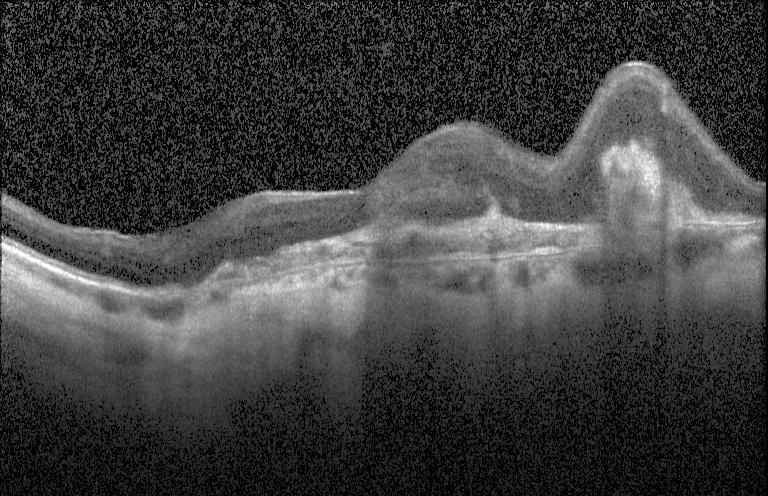
Impression: a choroidal neovascular membrane.